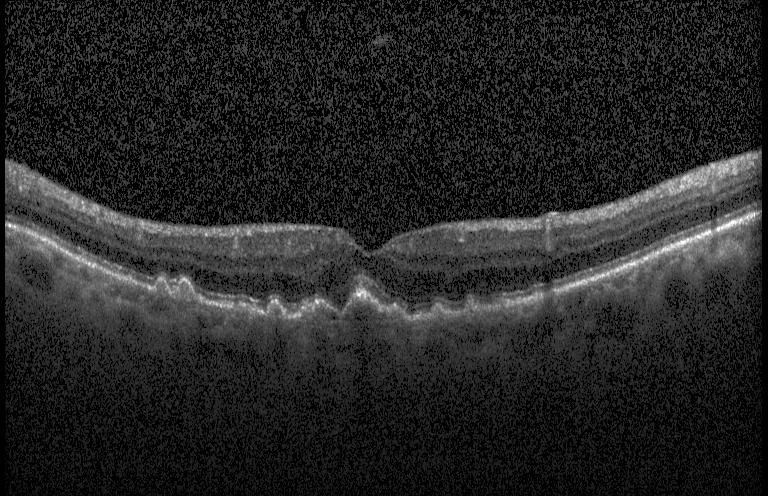
OCT line scan
The scan shows drusen.